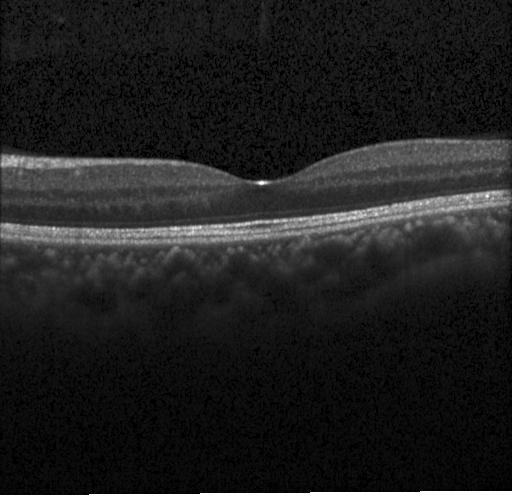
OCT B-scan.
Macular OCT: no CNV, DME, or drusen.